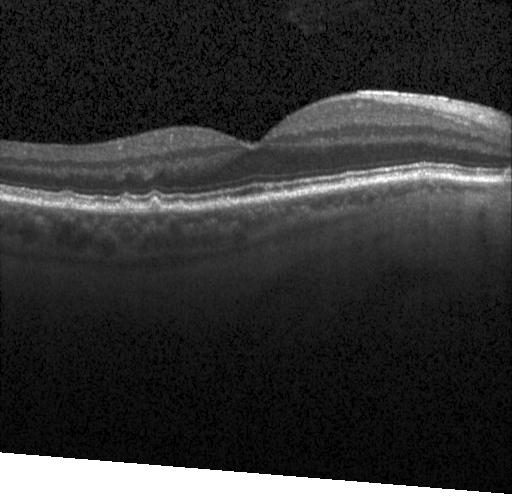

Heidelberg Spectralis; optical coherence tomography B-scan; spectral-domain OCT.
Dx: multiple drusen.